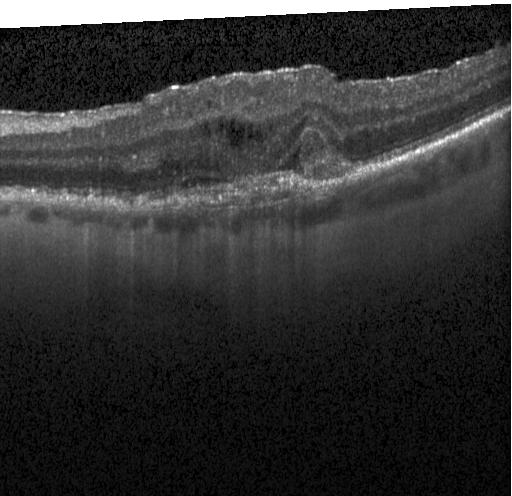

Spectral-domain OCT · instrument: Heidelberg Spectralis · retinal OCT B-scan · horizontal scan through the fovea — Diagnosis: CNV.